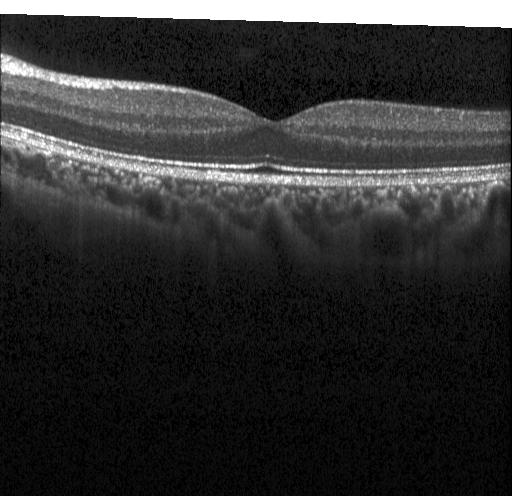 Horizontal scan through the fovea · optical coherence tomography B-scan.
Assessment: no choroidal neovascularization, no diabetic macular edema, and no drusen.